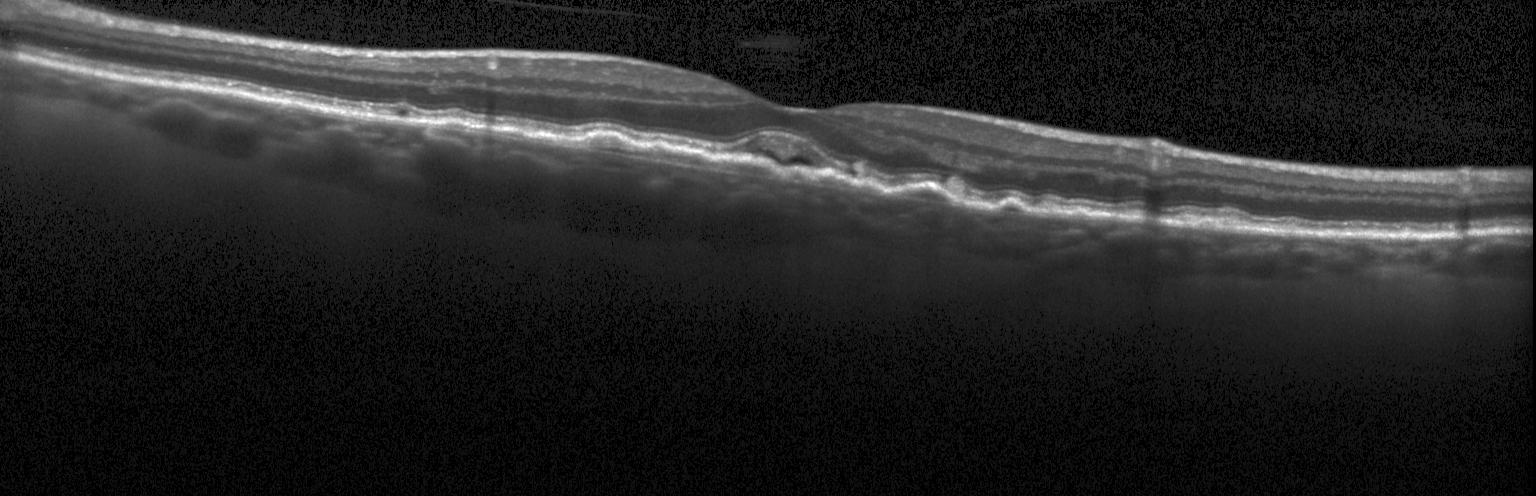 Macular scan; OCT line scan; spectral-domain optical coherence tomography; instrument: Heidelberg Spectralis. This B-scan demonstrates choroidal neovascularization.